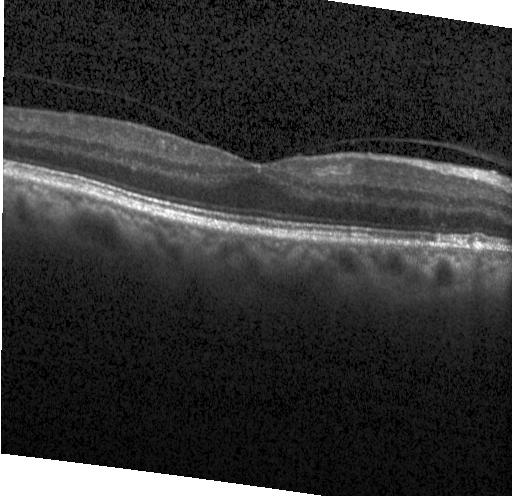 OCT B-scan showing multiple drusen.